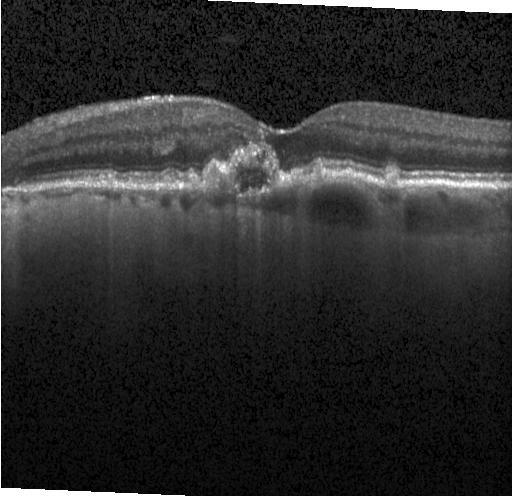

OCT line scan. Spectral-domain optical coherence tomography. Diagnosis: CNV.